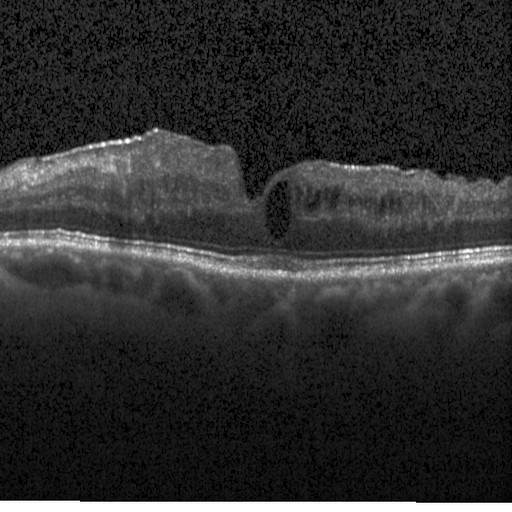
Diagnosis: DME.